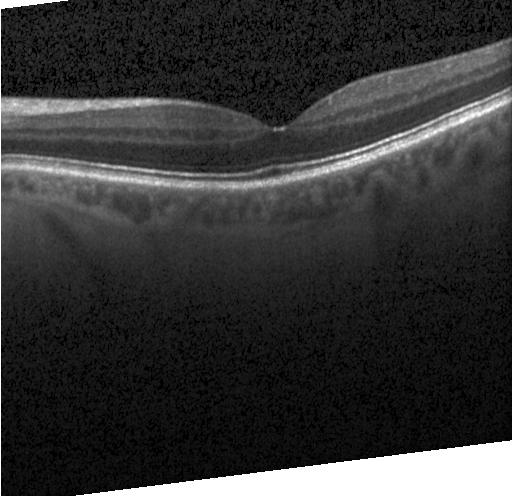 Retinal OCT cross-section — Finding: no CNV, DME, or drusen.